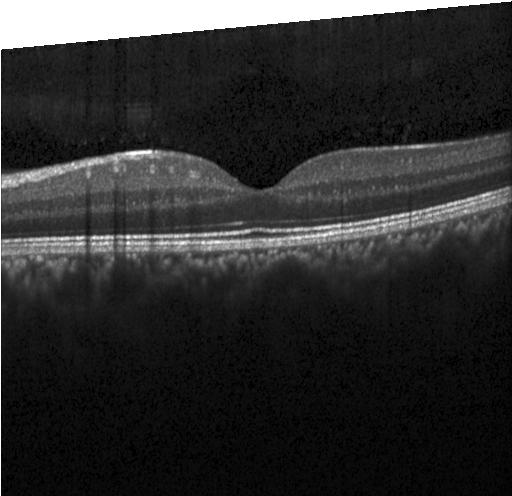

Spectral-domain OCT B-scan: no choroidal neovascularization, no diabetic macular edema, and no drusen.